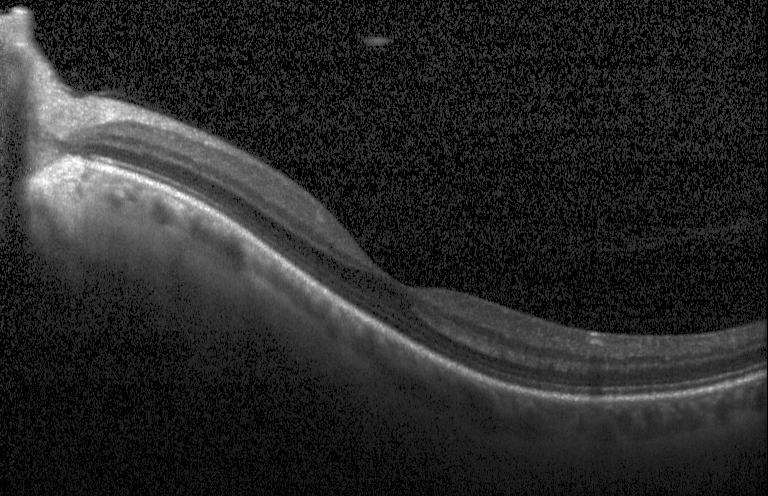 Heidelberg Spectralis OCT system · centered on the fovea · spectral-domain optical coherence tomography · OCT B-scan.
OCT finding: no evidence of choroidal neovascularization, diabetic macular edema, or drusen.